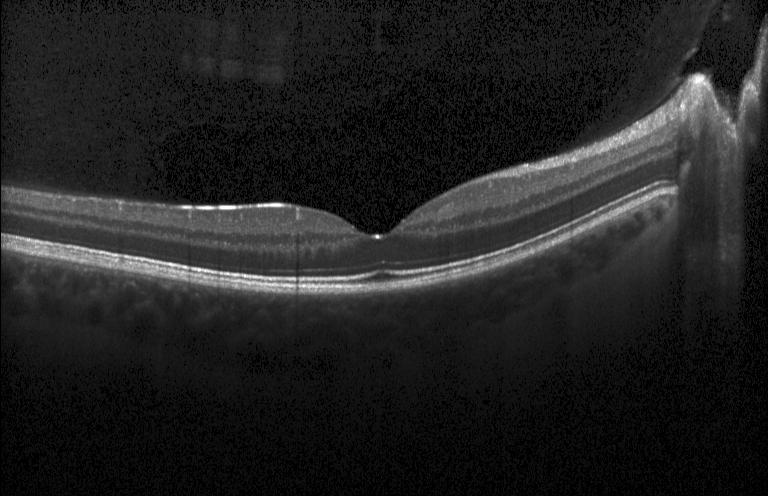
Horizontal scan through the fovea. Heidelberg Spectralis. SD-OCT. Optical coherence tomography scan.
OCT finding: no evidence of choroidal neovascularization, diabetic macular edema, or drusen.